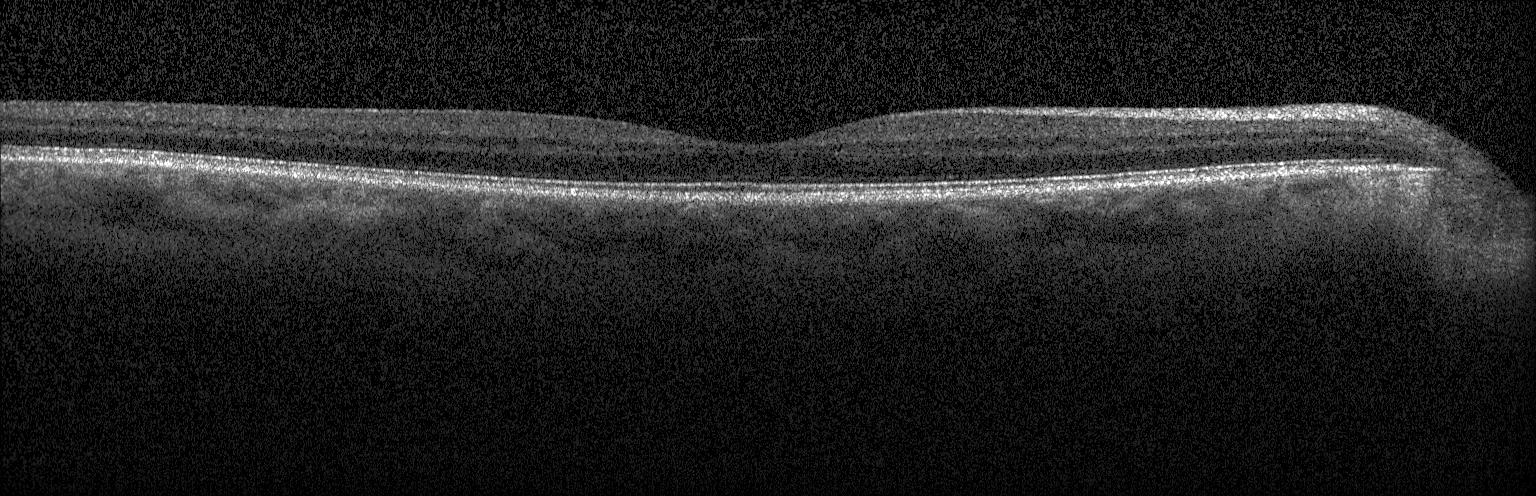 Spectral-domain OCT · optical coherence tomography B-scan.
OCT finding: no choroidal neovascularization, diabetic macular edema, or drusen.